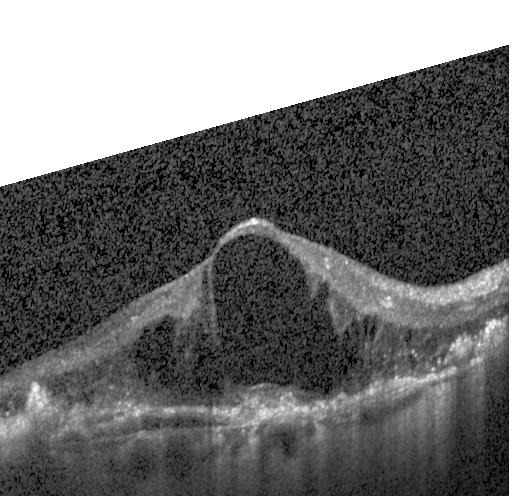 Assessment: CNV.